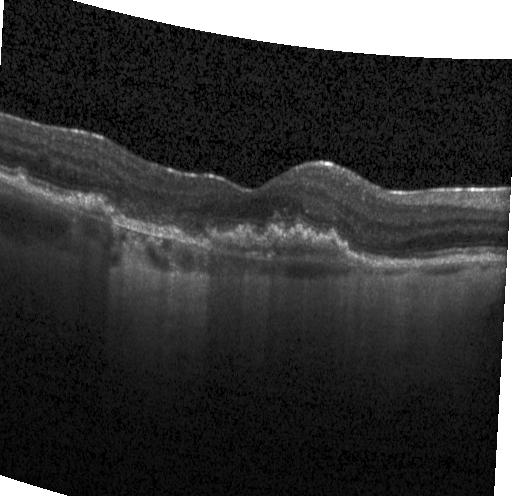 Macular OCT demonstrating choroidal neovascularization.